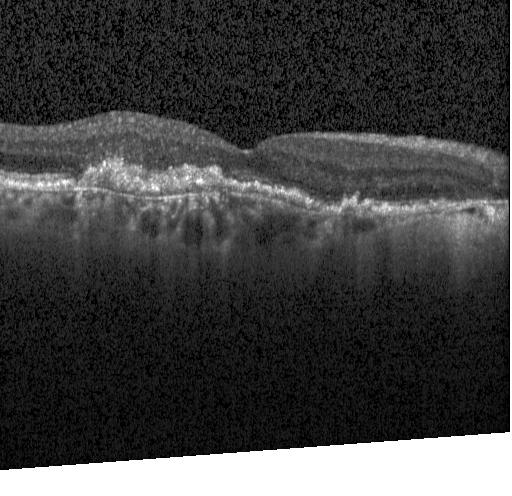
OCT line scan
Finding: a choroidal neovascular membrane.